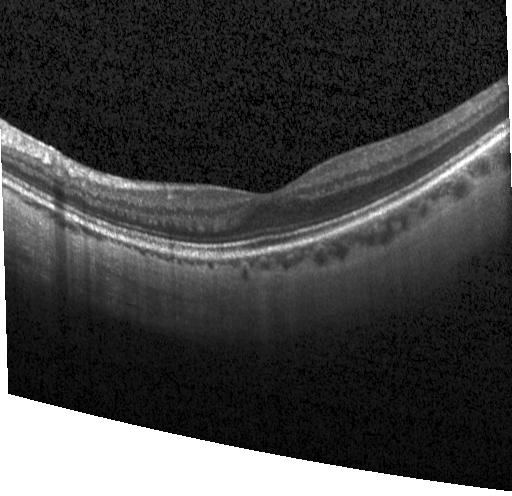
Optical coherence tomography B-scan; SD-OCT; centered on the fovea. Impression: no evidence of choroidal neovascularization, diabetic macular edema, or drusen.